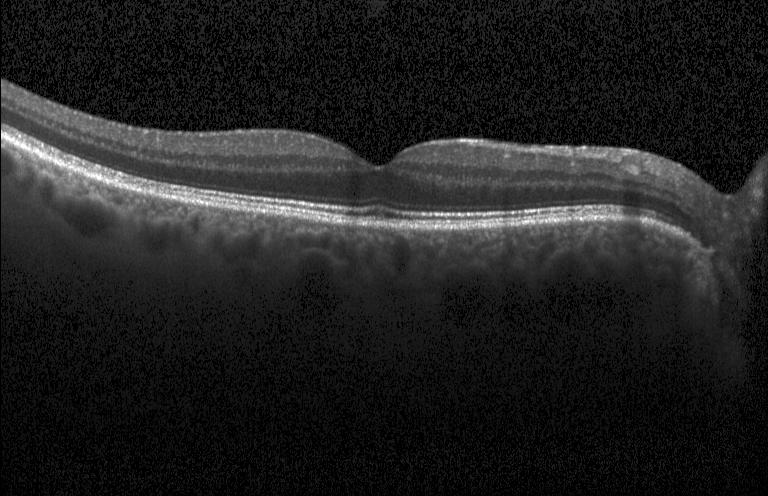
OCT B-scan showing no evidence of CNV, DME, or drusen.